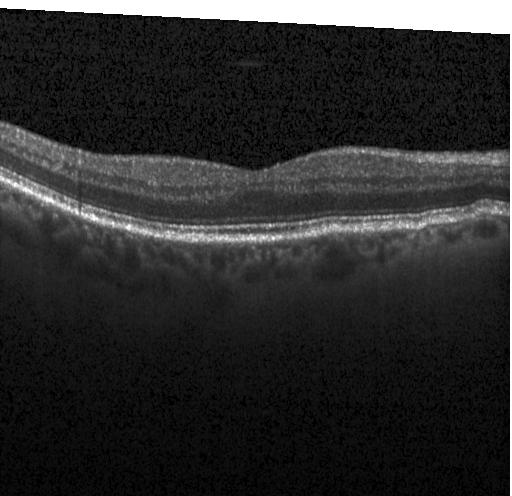 Diagnosis: no evidence of CNV, DME, or drusen.